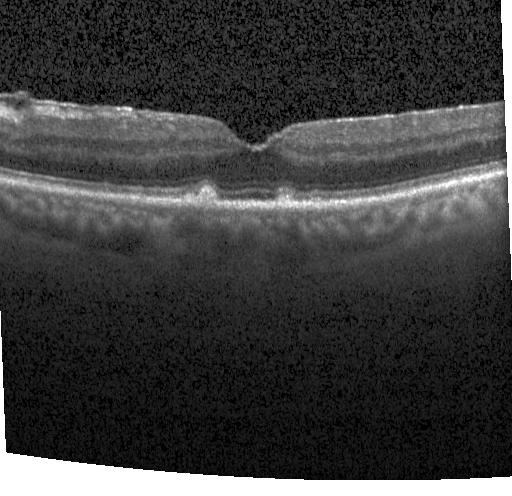
This B-scan demonstrates drusen.